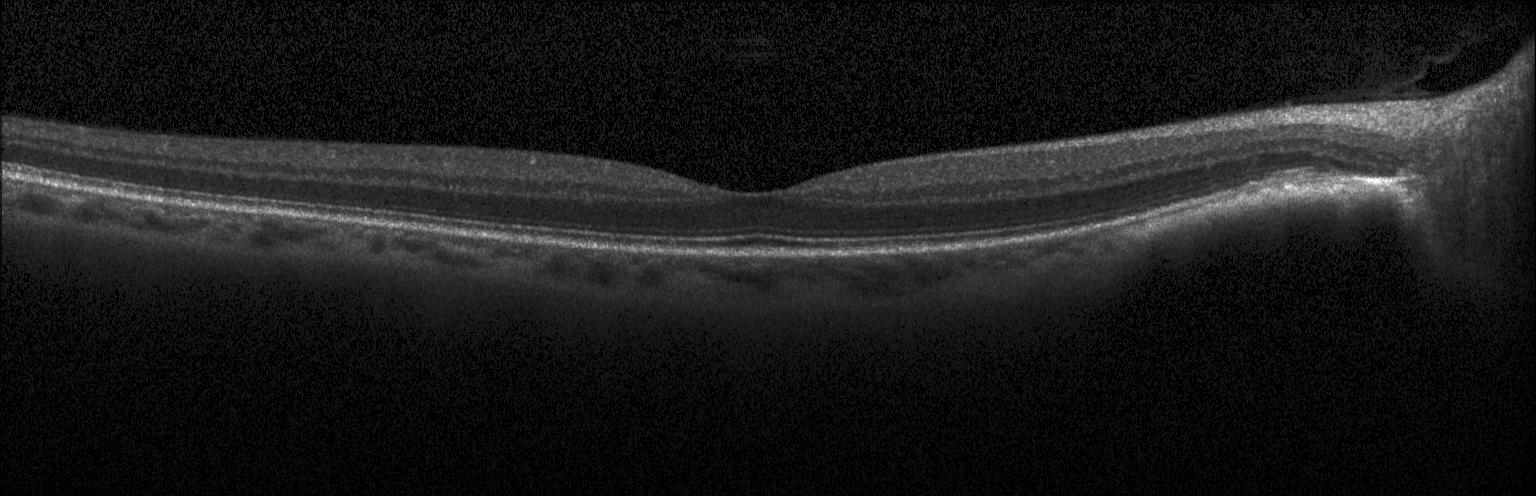
Spectral-domain OCT B-scan: neither CNV, DME, nor drusen.